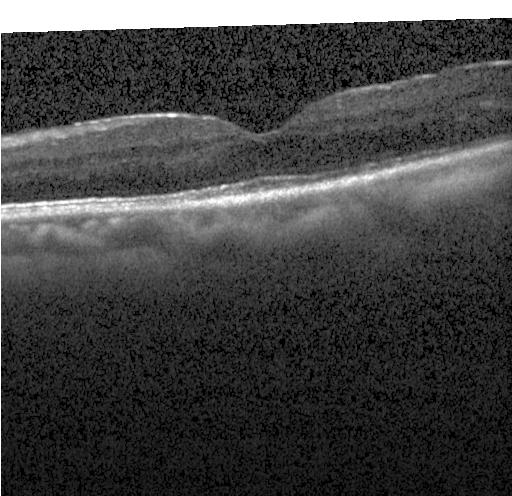

Heidelberg Spectralis OCT system. Macular scan. OCT B-scan.
Diagnosis: no evidence of choroidal neovascularization, diabetic macular edema, or drusen.